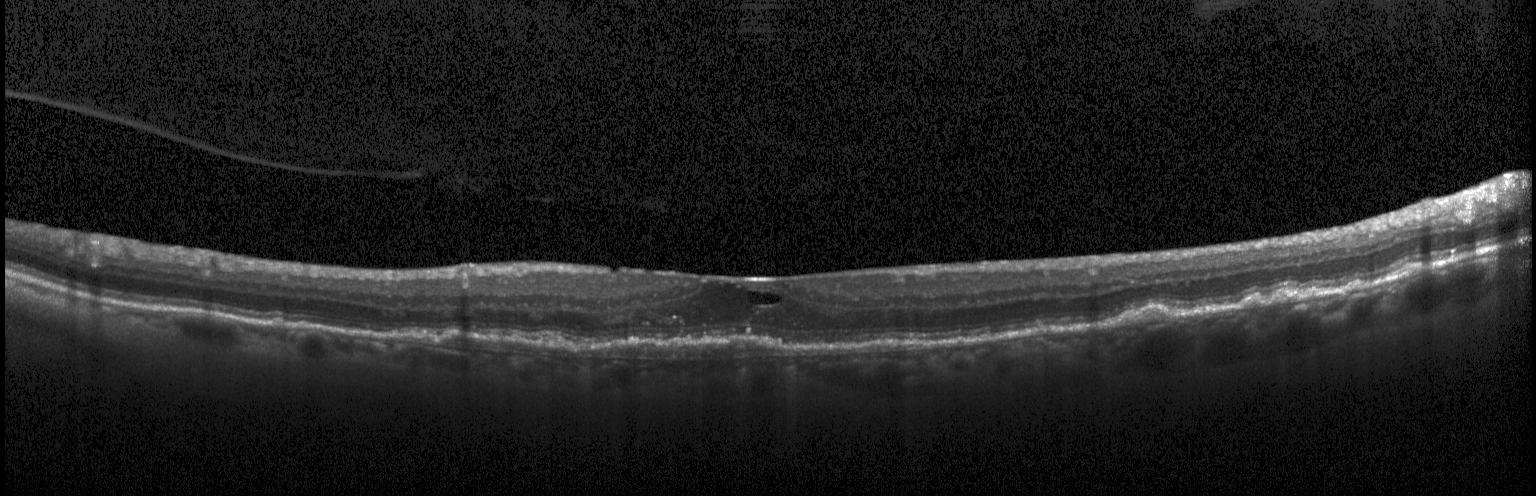 Assessment: a choroidal neovascular membrane.